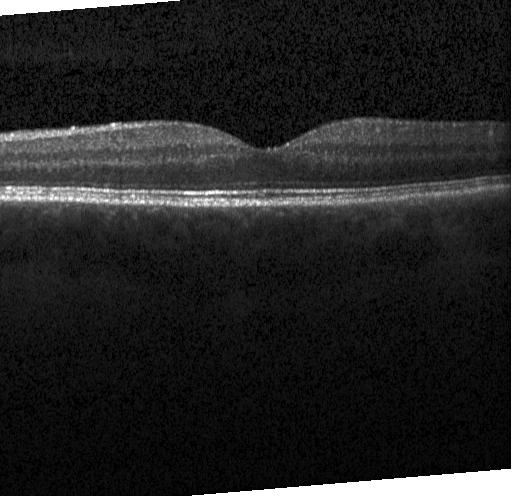 Dx: neither CNV, DME, nor drusen.